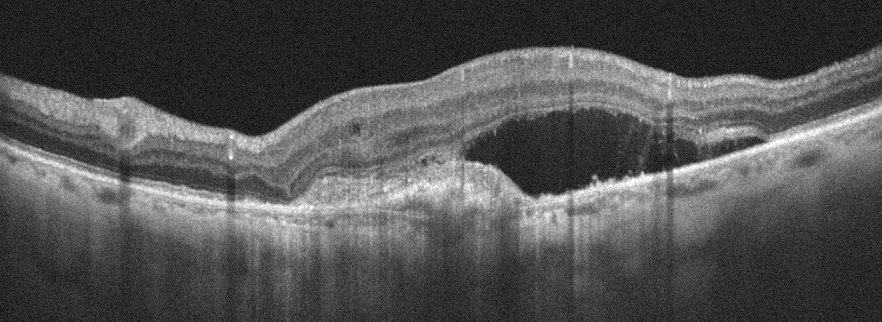
Oculus sinister · OCT line scan.
Impression: age-related macular degeneration.